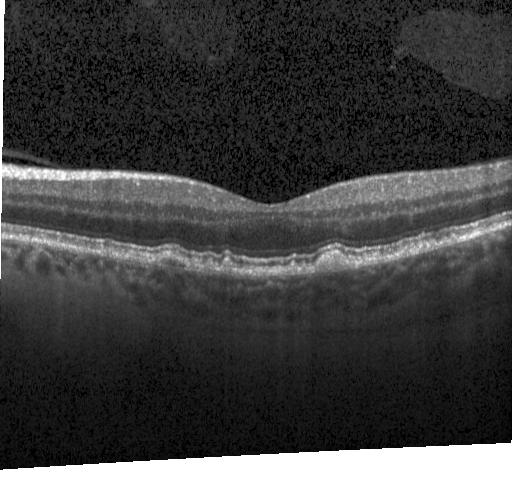

Optical coherence tomography scan.
Diagnosis: multiple drusen.